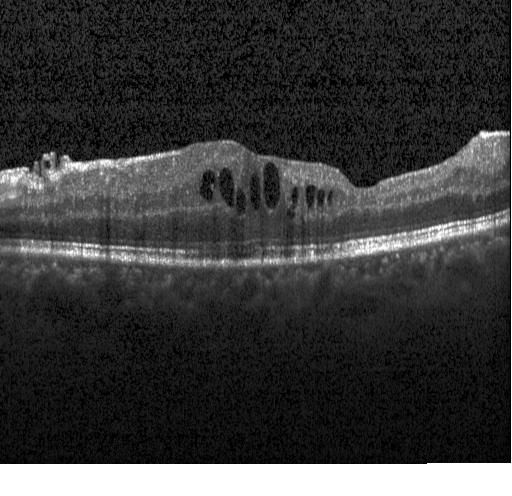 Optical coherence tomography scan; macular scan
Diagnosis: diabetic macular edema (DME).